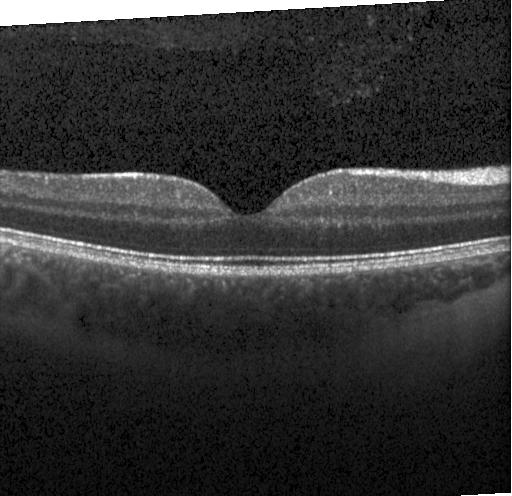 Impression: neither choroidal neovascularization, diabetic macular edema, nor drusen.